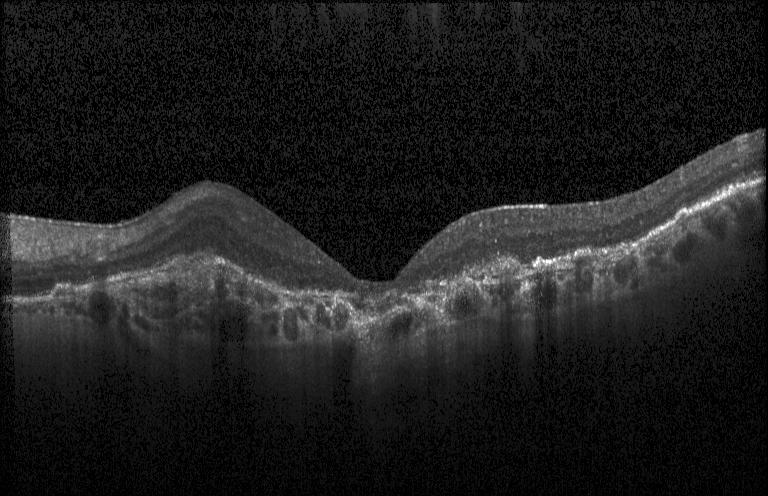 Horizontal scan through the fovea. OCT B-scan.
Dx: choroidal neovascularization.